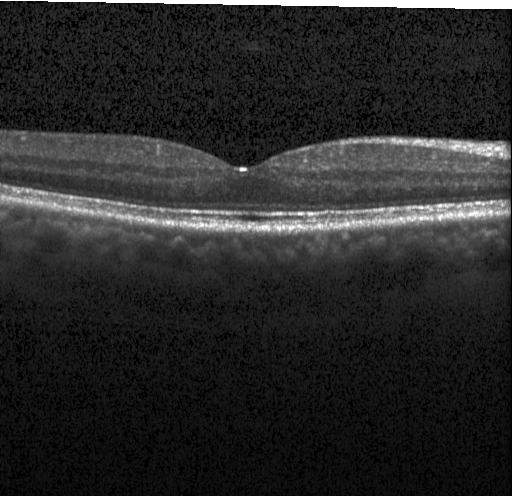 OCT line scan, centered on the fovea, SD-OCT — Finding: no choroidal neovascularization, diabetic macular edema, or drusen.